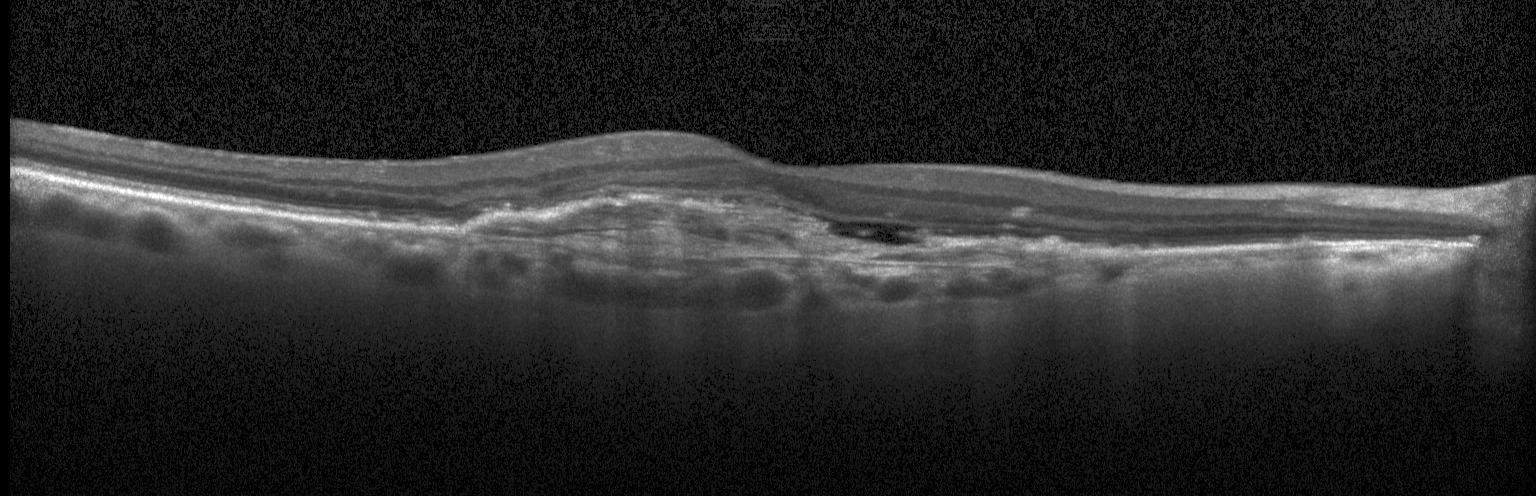
Retinal OCT B-scan · macular scan — Assessment: a choroidal neovascular membrane.